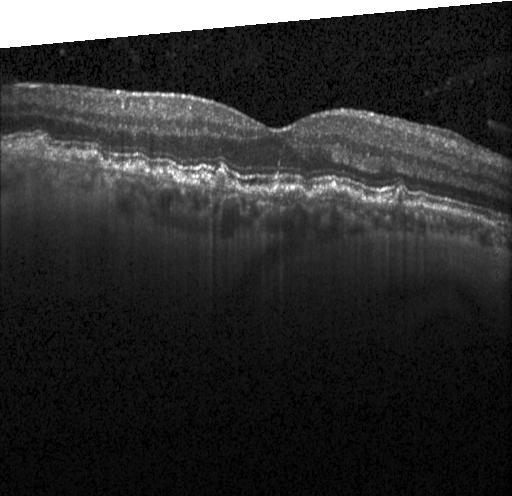 OCT B-scan; SD-OCT.
Finding: sub-RPE drusenoid deposits.